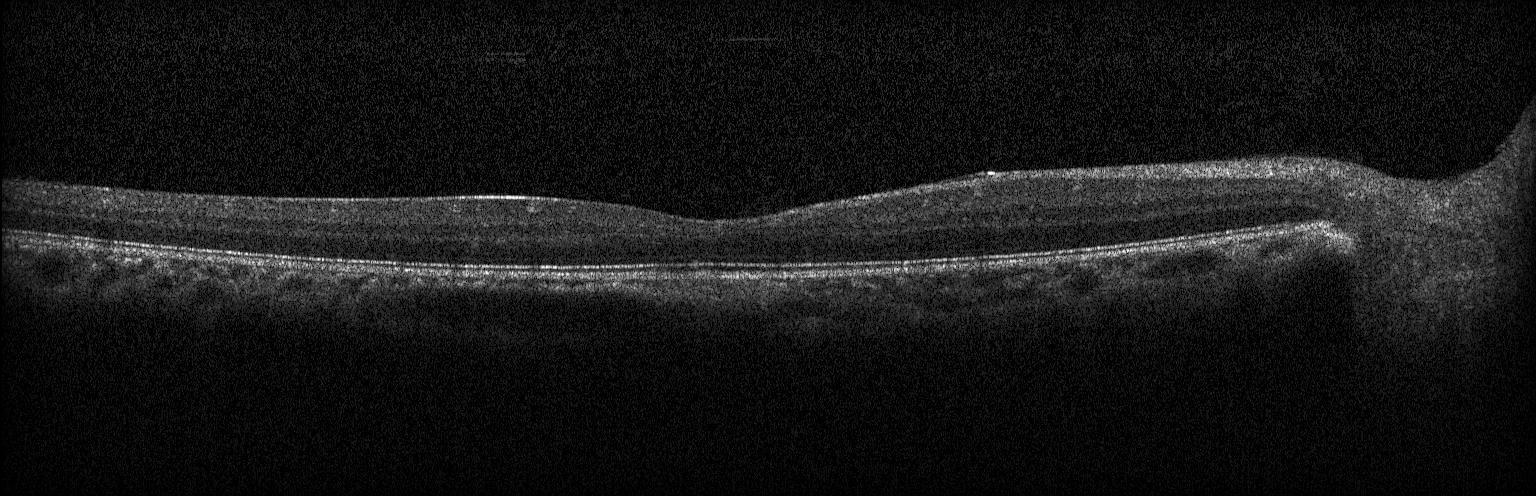
Impression: no choroidal neovascularization, no diabetic macular edema, and no drusen.